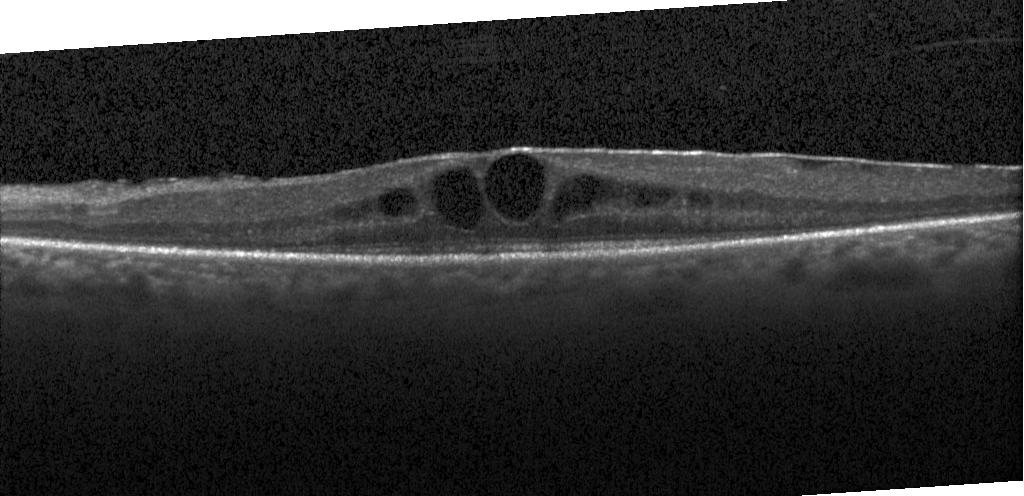
This B-scan demonstrates diabetic macular edema (DME).